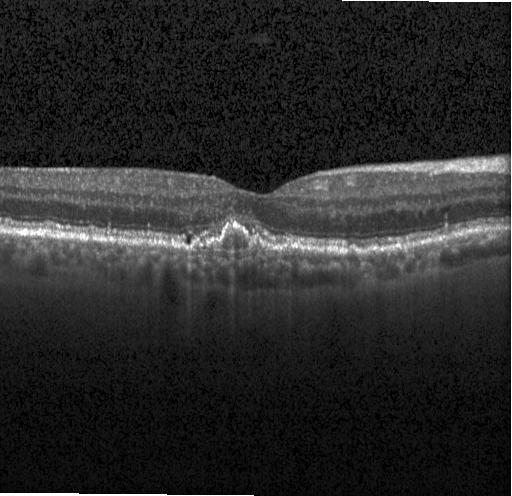

The scan shows a choroidal neovascular membrane.